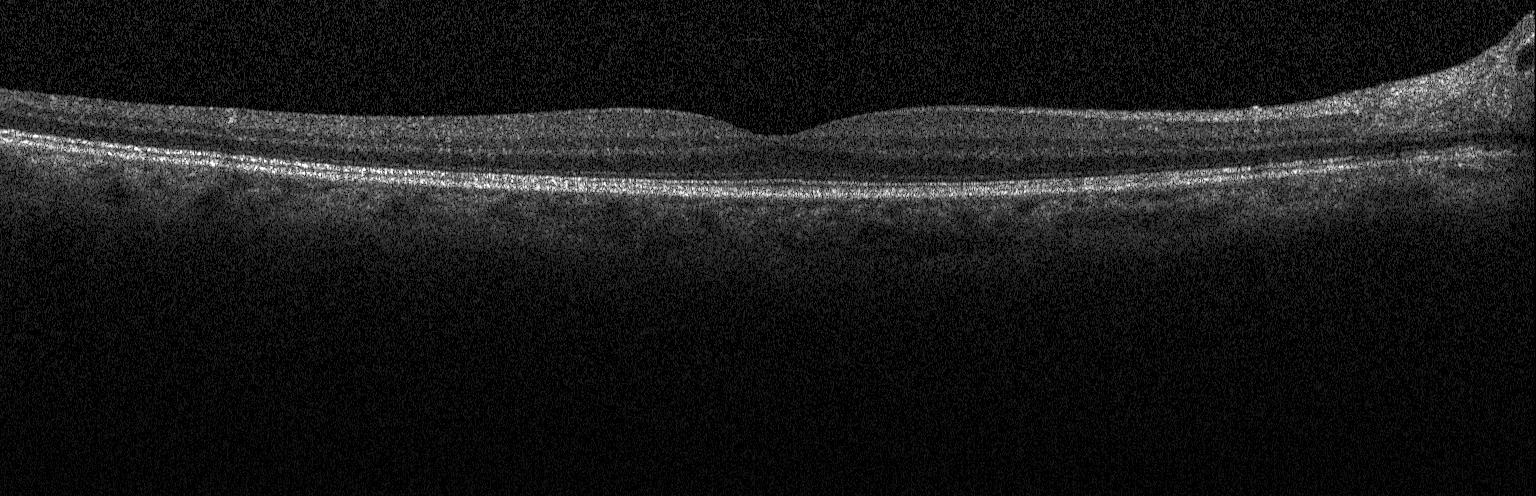

OCT B-scan showing neither CNV, DME, nor drusen.